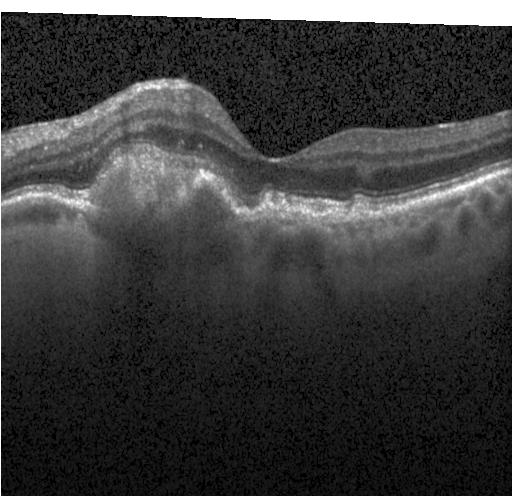 Finding: a choroidal neovascular membrane.